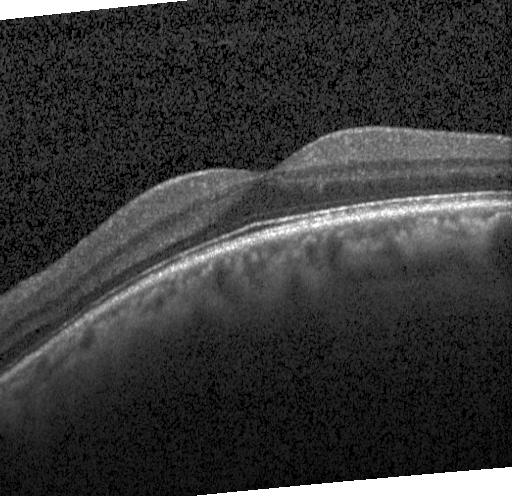 Impression: neither choroidal neovascularization, diabetic macular edema, nor drusen.